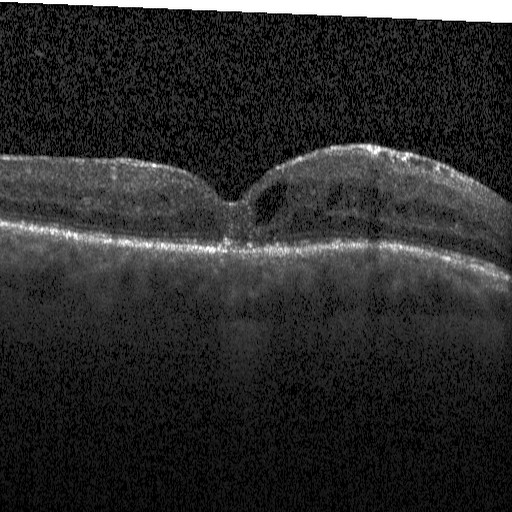
OCT scan showing DME.